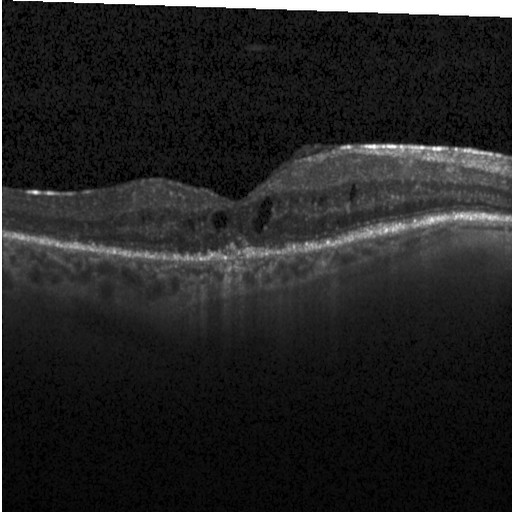 Centered on the fovea · OCT line scan.
Finding: DME.